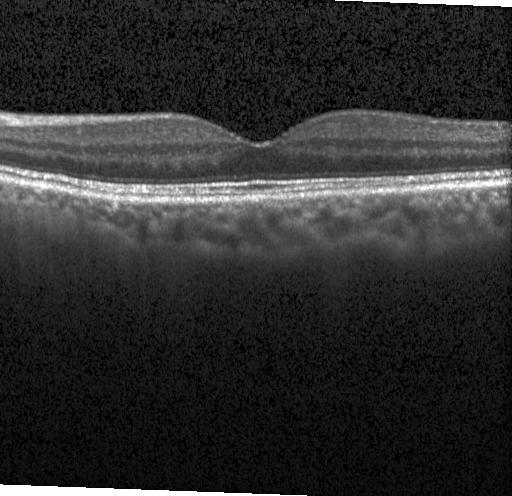 Optical coherence tomography B-scan. Impression: no choroidal neovascularization, diabetic macular edema, or drusen.